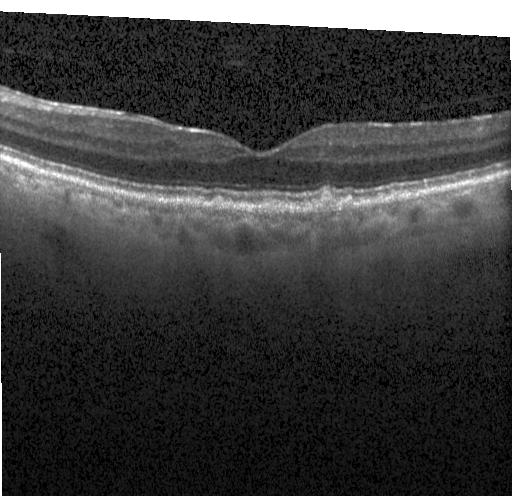 Assessment: multiple drusen.